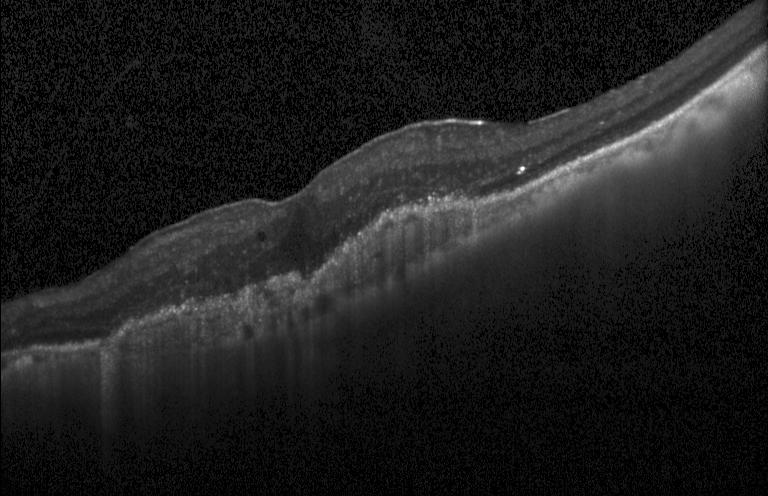

Dx: choroidal neovascularization.